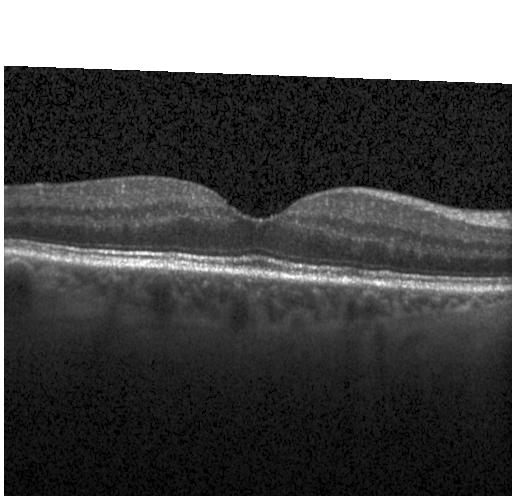 Diagnosis: no choroidal neovascularization, no diabetic macular edema, and no drusen.